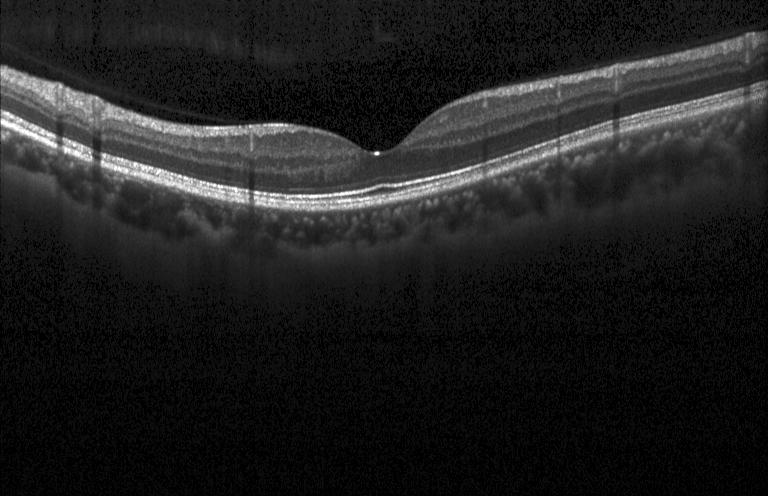 SD-OCT. Optical coherence tomography B-scan. Heidelberg Spectralis OCT system
Macular OCT: no CNV, no DME, and no drusen.